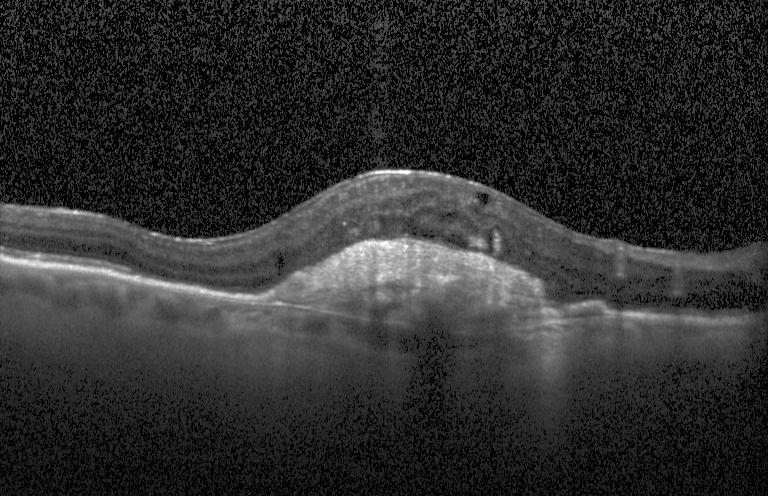

Diagnosis: CNV.